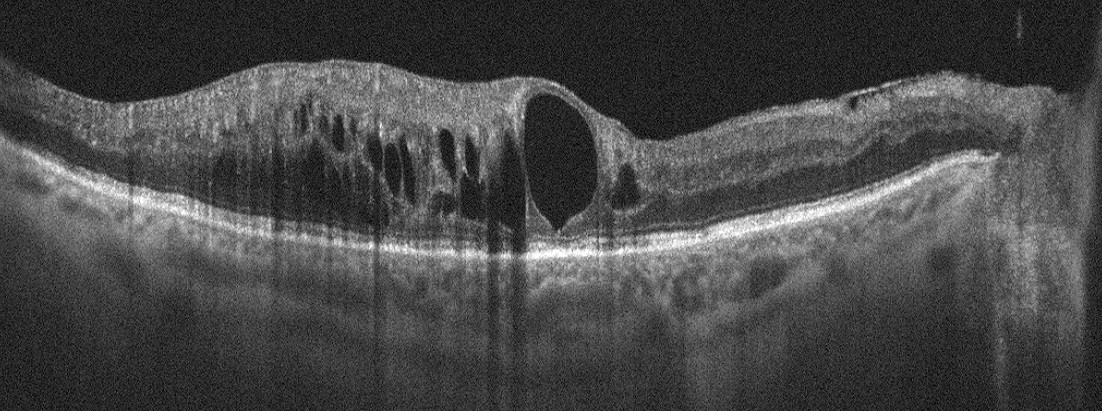

Optovue Avanti RTVue XR, retinal OCT B-scan, fovea-centered.
Impression: diabetic macular edema.